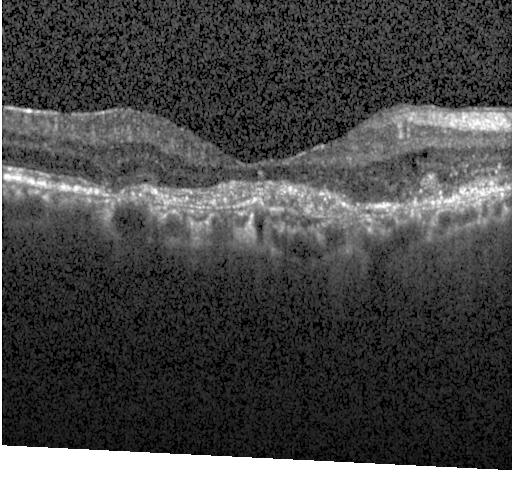 Diagnosis: CNV.